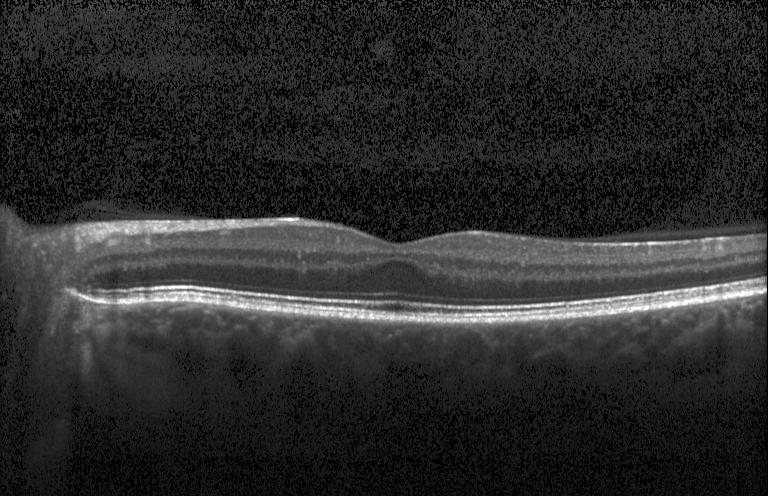
Optical coherence tomography B-scan; through the macula; spectral-domain optical coherence tomography; Heidelberg Spectralis
The scan shows neither choroidal neovascularization, diabetic macular edema, nor drusen.